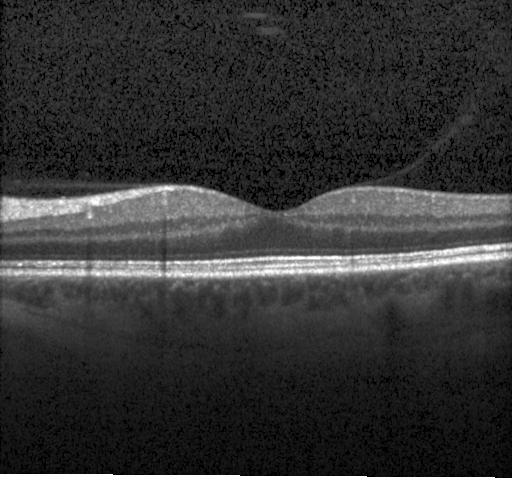 Macular scan. Optical coherence tomography B-scan
Macular OCT: no choroidal neovascularization, no diabetic macular edema, and no drusen.